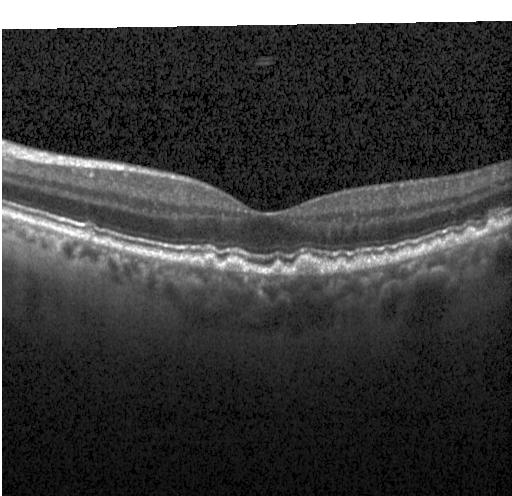 Diagnosis: multiple drusen.